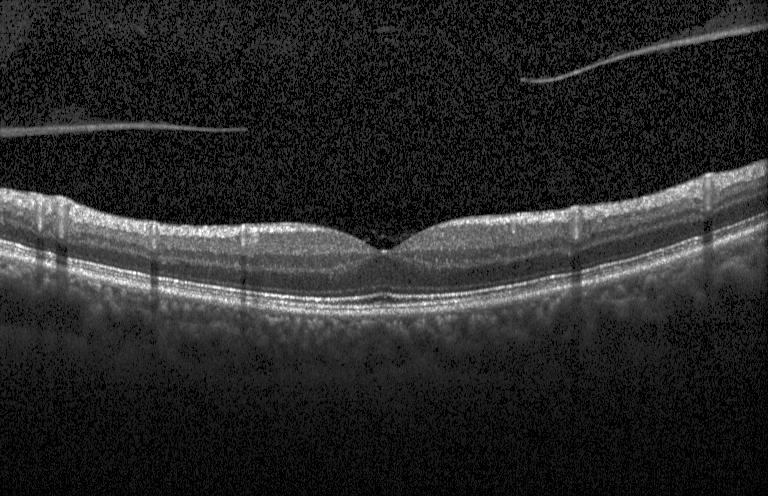 SD-OCT; through the macula; instrument: Heidelberg Spectralis; optical coherence tomography scan
The scan shows no evidence of choroidal neovascularization, diabetic macular edema, or drusen.